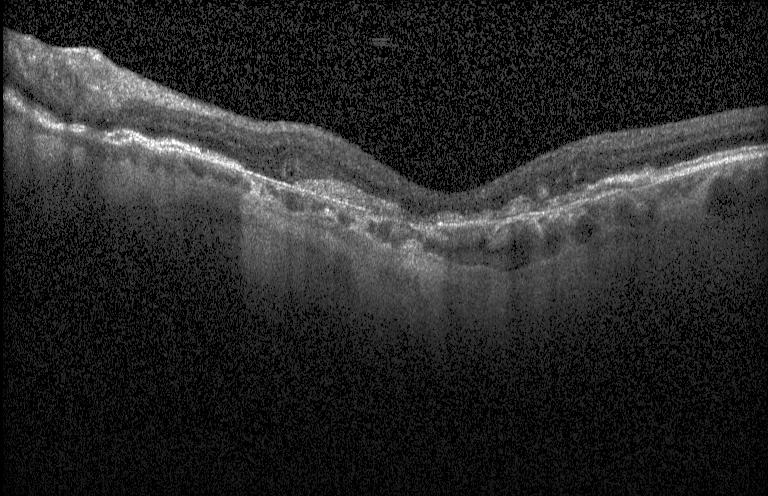

Acquired on a Heidelberg Spectralis. OCT line scan. Macular scan. Spectral-domain optical coherence tomography
This B-scan demonstrates a choroidal neovascular membrane.